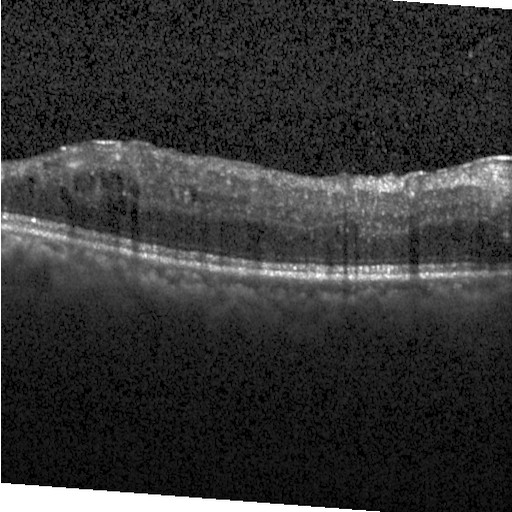
Retinal OCT B-scan.
Finding: diabetic macular edema.